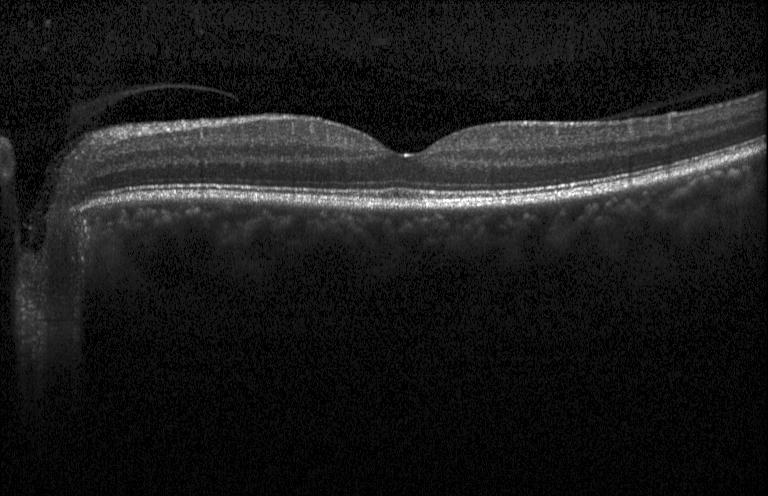
Assessment: no choroidal neovascularization, no diabetic macular edema, and no drusen.